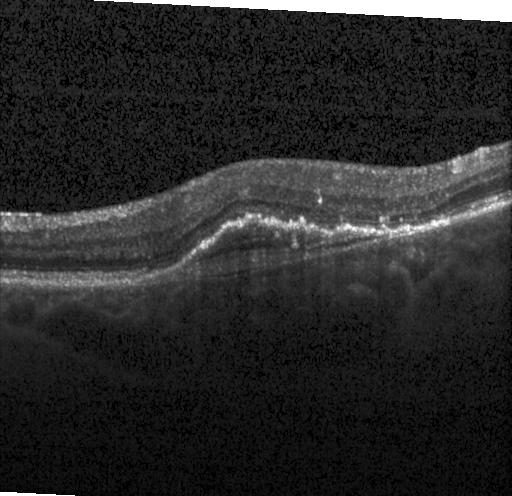 Assessment: a choroidal neovascular membrane.